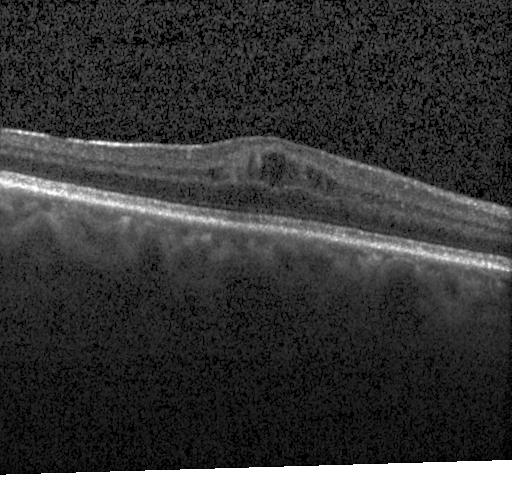
Spectral-domain optical coherence tomography; instrument: Heidelberg Spectralis; centered on the fovea; optical coherence tomography B-scan
Finding: diabetic macular edema (DME).